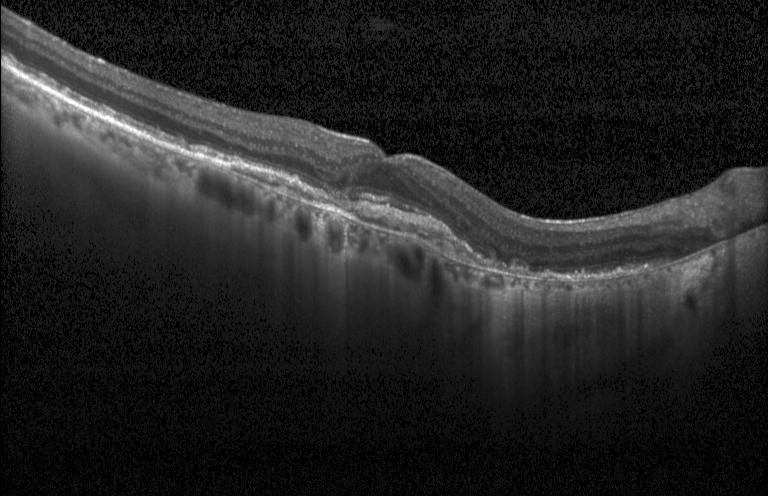 A choroidal neovascular membrane.